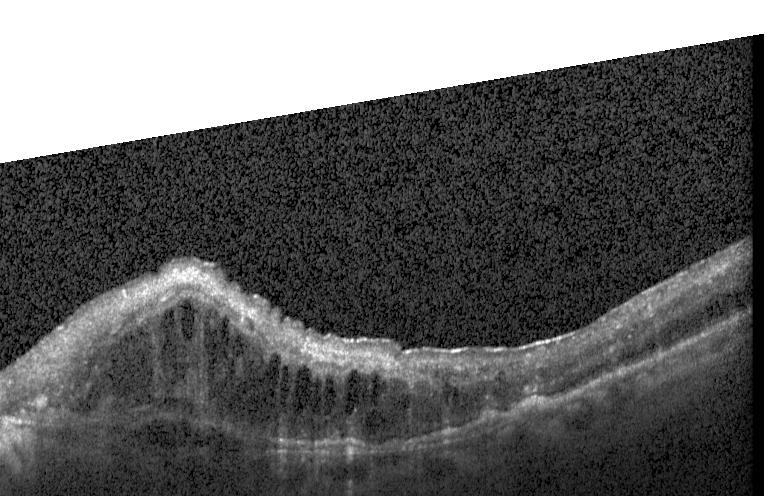
Spectral-domain optical coherence tomography. Retinal OCT cross-section. Macular scan. This B-scan demonstrates choroidal neovascularization.